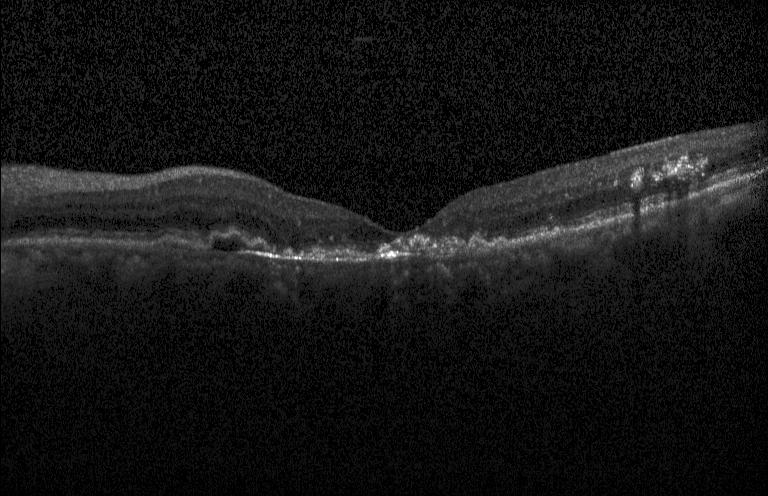
Optical coherence tomography scan. Spectral-domain OCT. Macular scan. Acquired on a Heidelberg Spectralis. OCT finding: CNV.